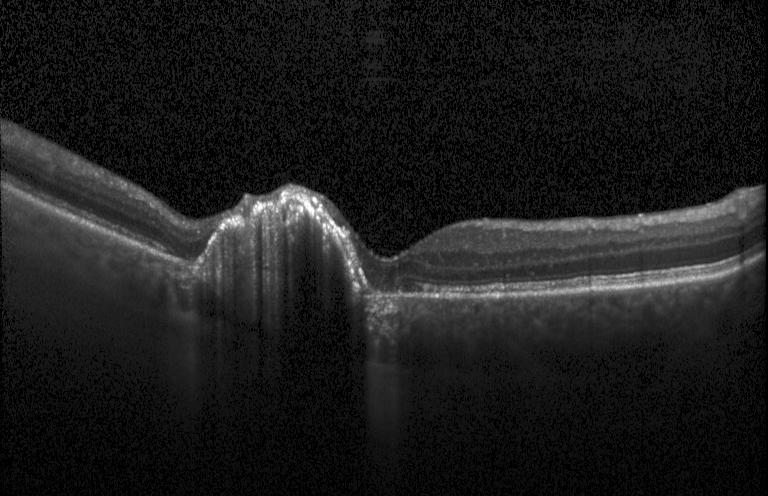

Optical coherence tomography scan
This B-scan demonstrates choroidal neovascularization (CNV).